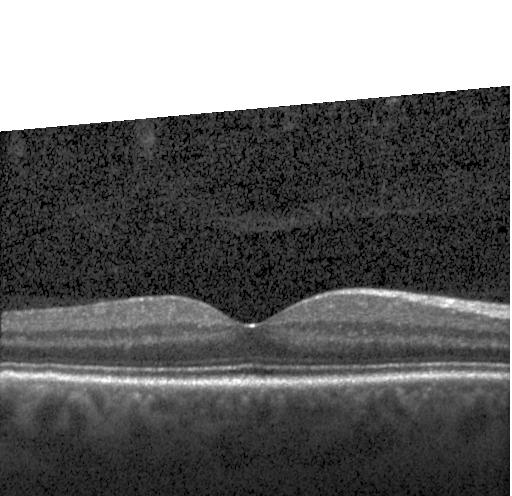 Assessment: no choroidal neovascularization, diabetic macular edema, or drusen.